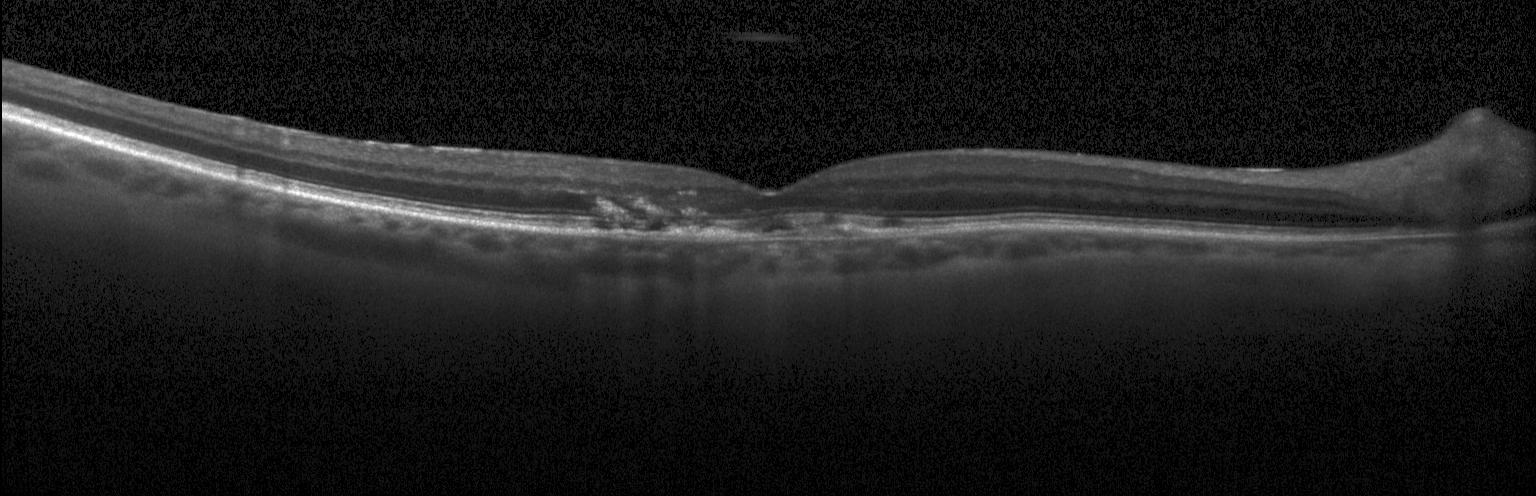 Optical coherence tomography B-scan, through the macula, SD-OCT.
Impression: choroidal neovascularization.